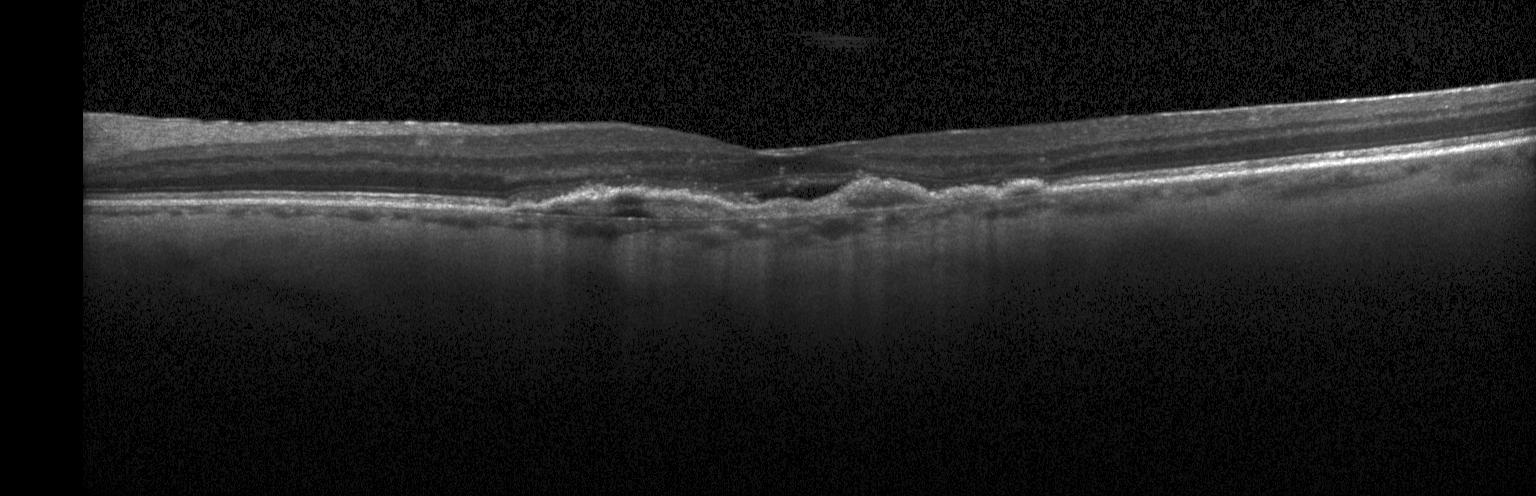

Centered on the fovea. OCT line scan. Spectral-domain optical coherence tomography — This B-scan demonstrates a choroidal neovascular membrane.